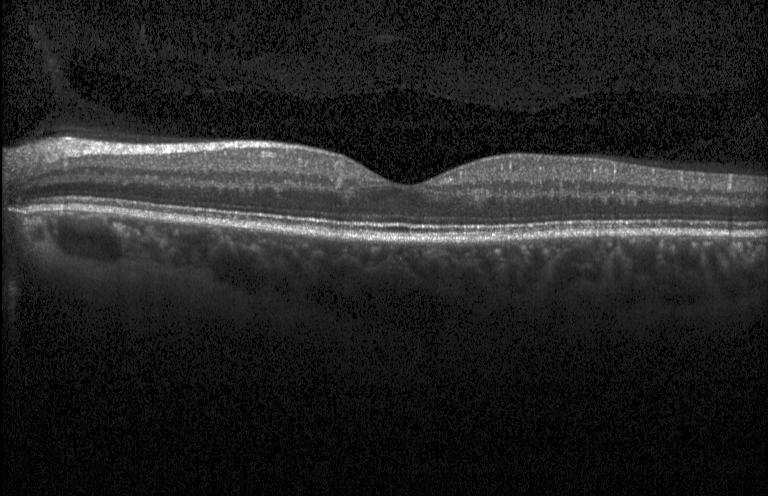 Spectral-domain OCT B-scan: neither CNV, DME, nor drusen.